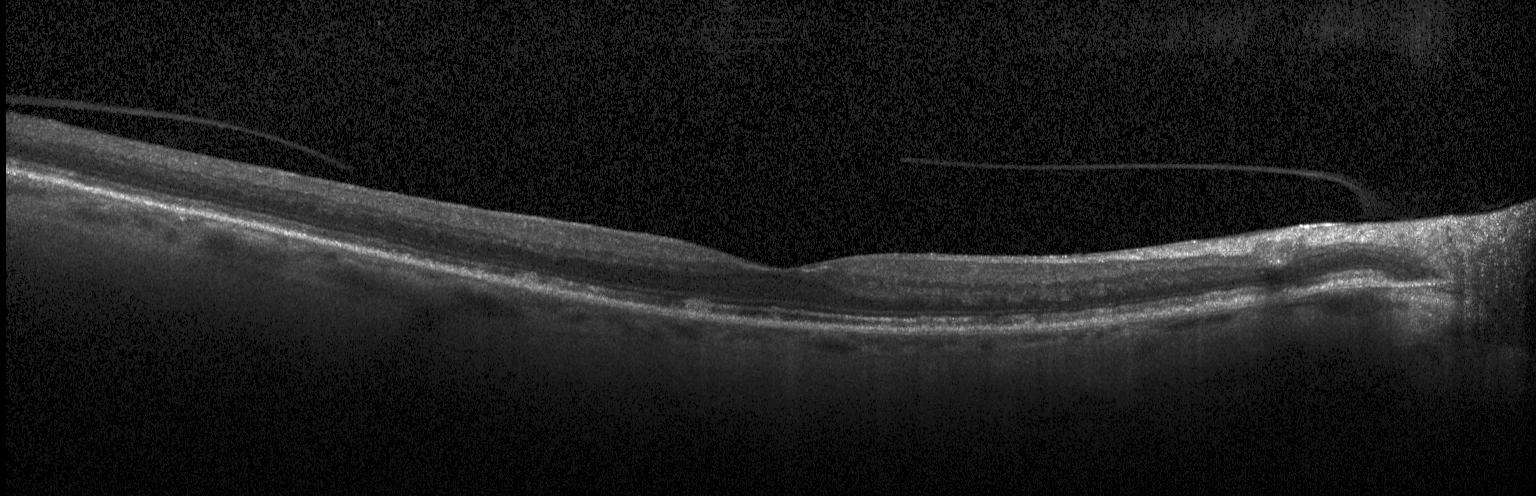

Fovea-centered, acquired on a Heidelberg Spectralis, optical coherence tomography B-scan — Finding: drusen.